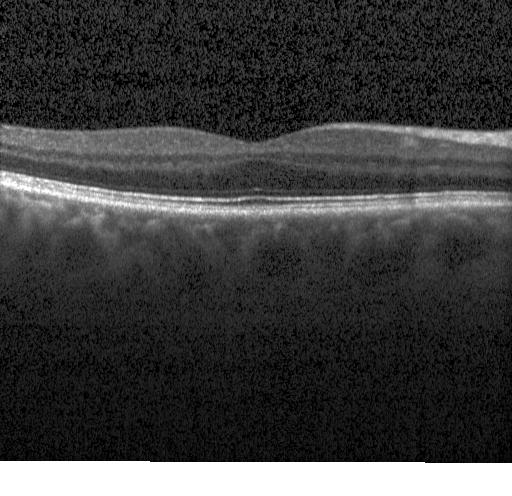
OCT line scan — This B-scan demonstrates no choroidal neovascularization, diabetic macular edema, or drusen.